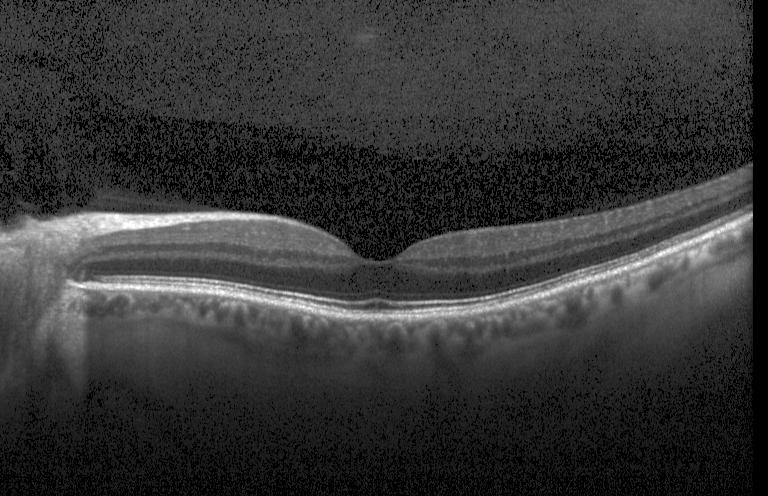

Optical coherence tomography scan — This B-scan demonstrates no evidence of choroidal neovascularization, diabetic macular edema, or drusen.